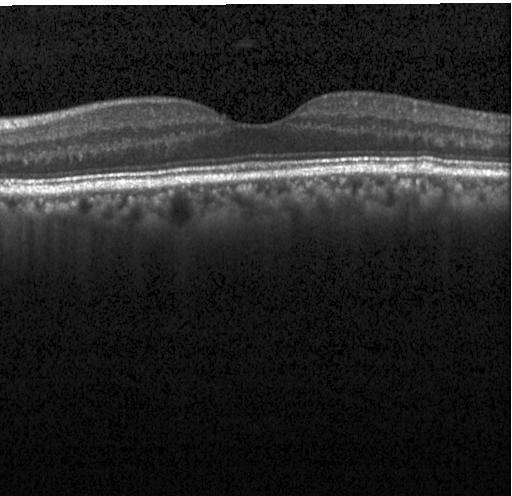 OCT line scan · spectral-domain OCT. Dx: no CNV, DME, or drusen.